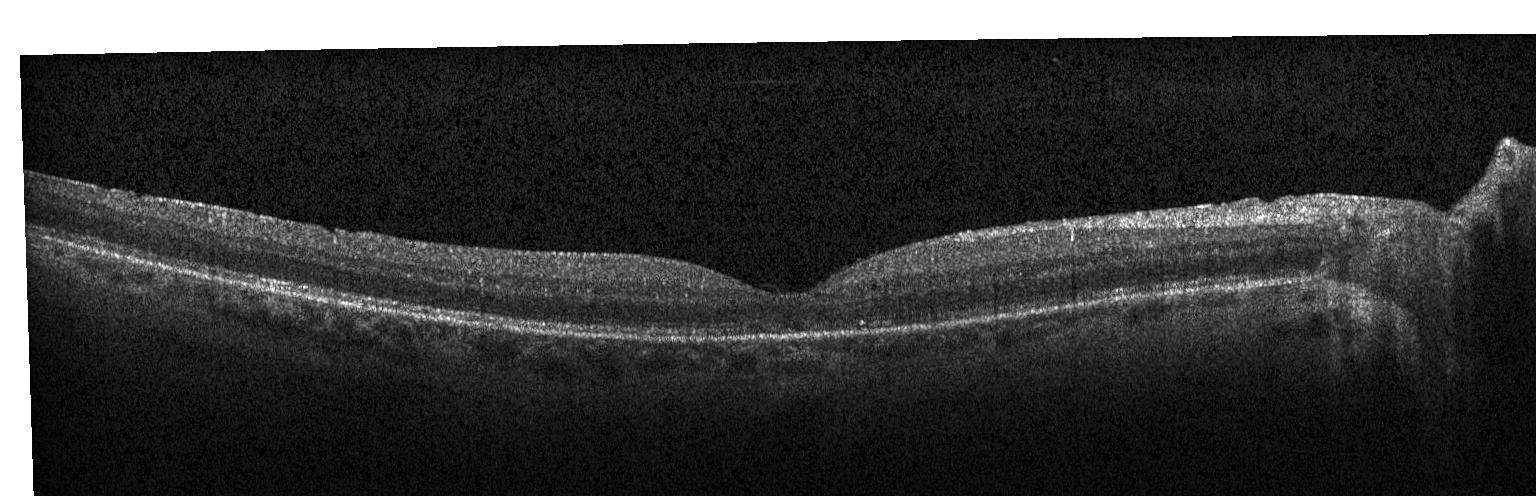 Finding: no evidence of choroidal neovascularization, diabetic macular edema, or drusen.